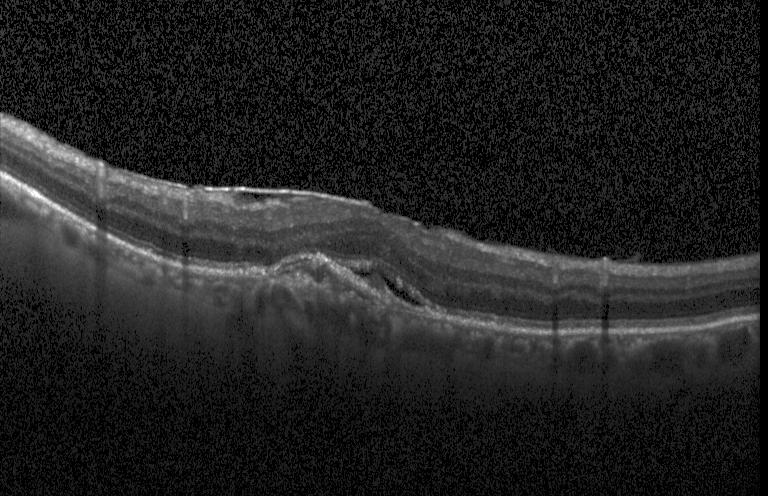
Finding: a choroidal neovascular membrane.